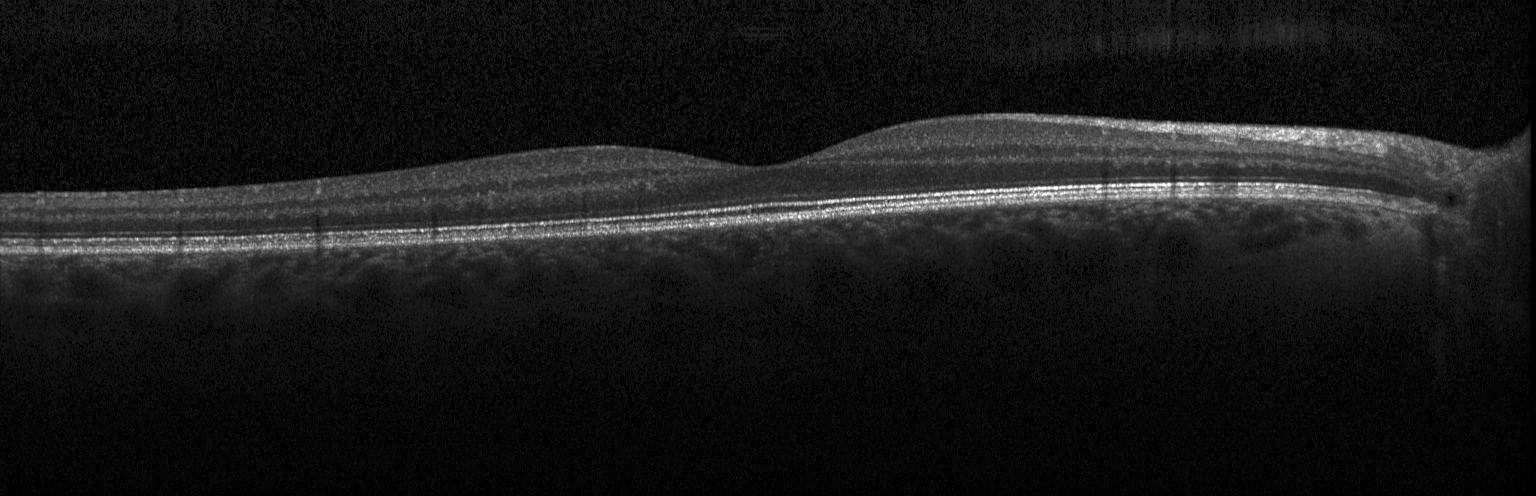 Spectral-domain OCT B-scan: neither CNV, DME, nor drusen.